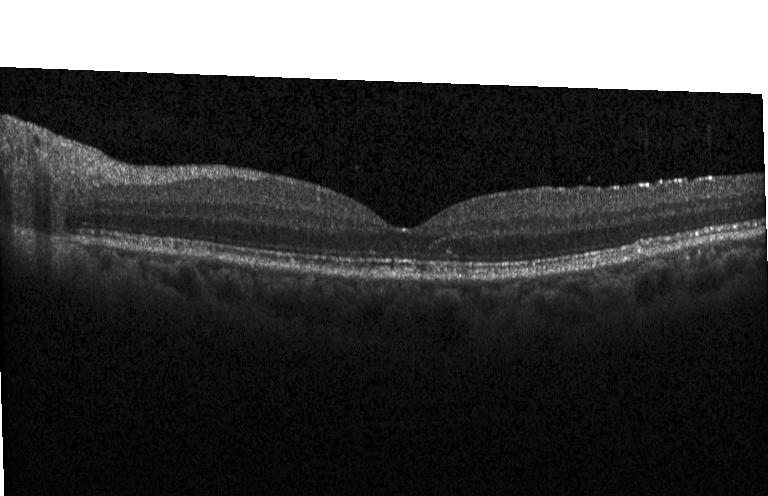 Macular OCT: no evidence of CNV, DME, or drusen.